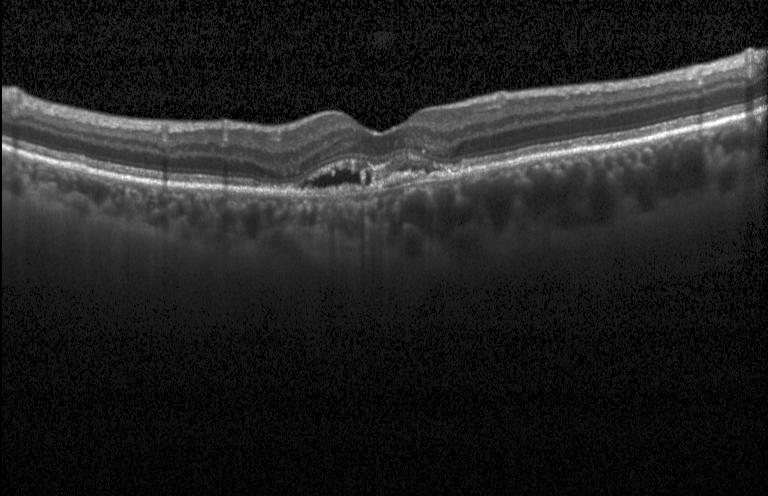
Optical coherence tomography B-scan. Diagnosis: choroidal neovascularization.